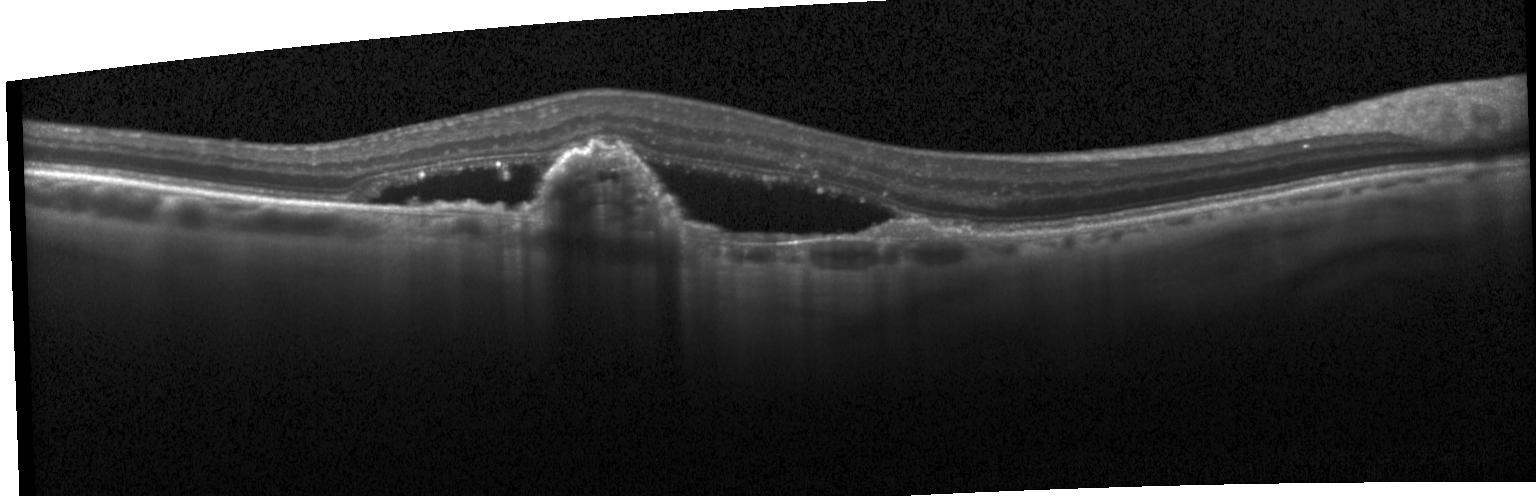

Dx: a choroidal neovascular membrane.